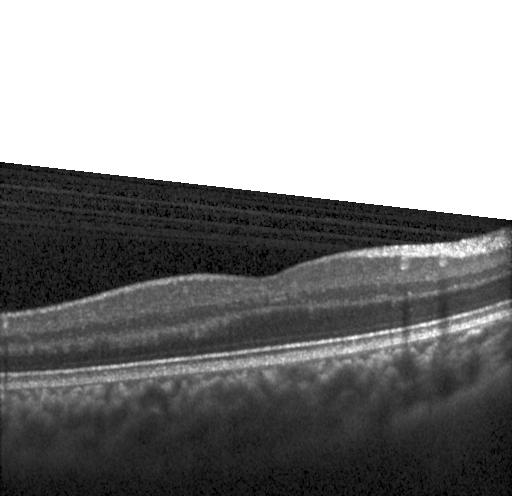 Optical coherence tomography B-scan — OCT finding: no evidence of CNV, DME, or drusen.